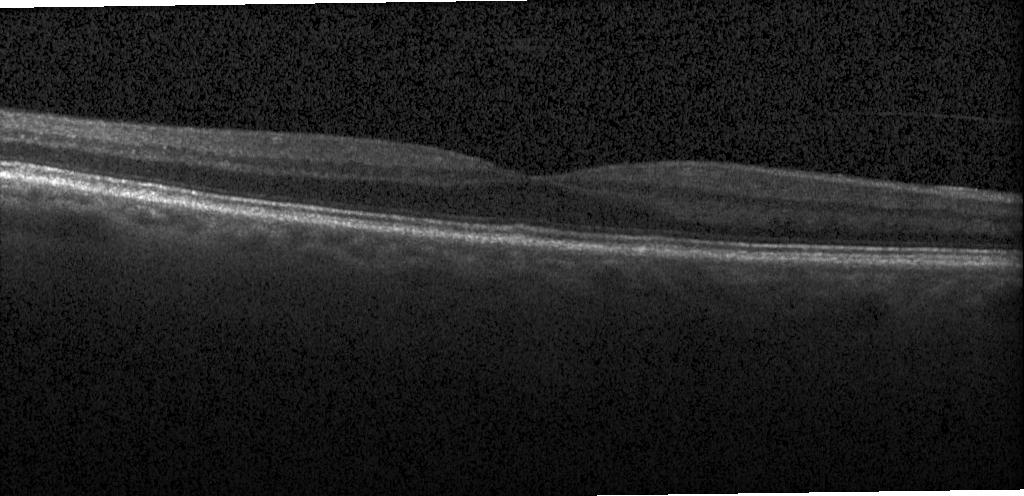 OCT line scan
Dx: no evidence of CNV, DME, or drusen.